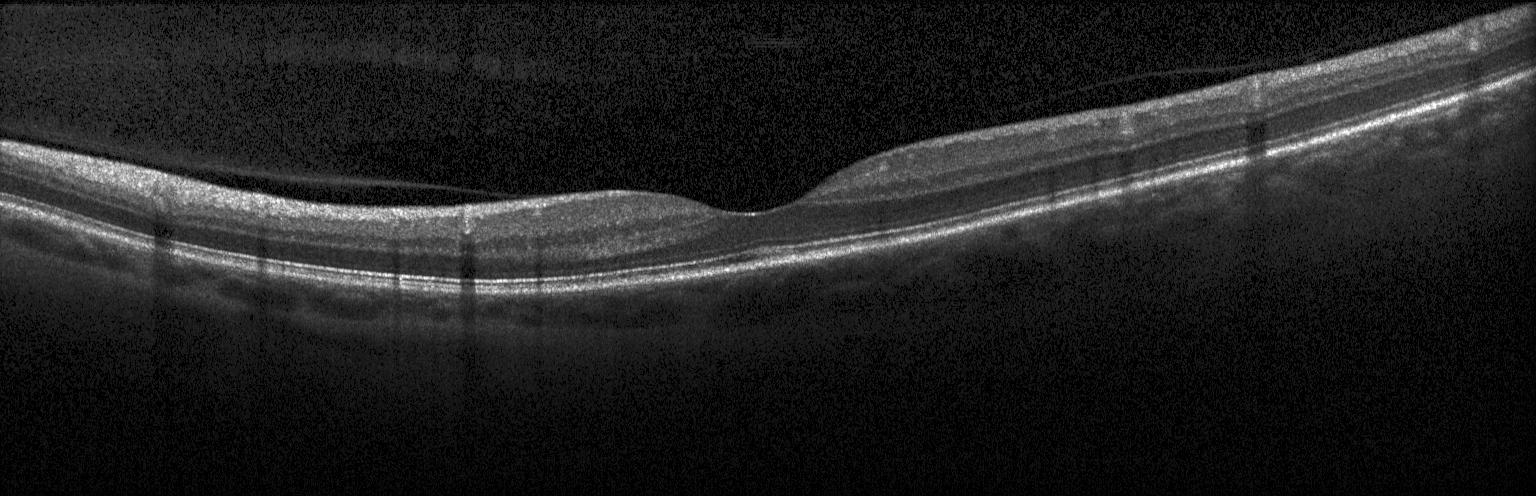 Spectral-domain OCT. Heidelberg Spectralis OCT system. OCT line scan
No evidence of choroidal neovascularization, diabetic macular edema, or drusen.